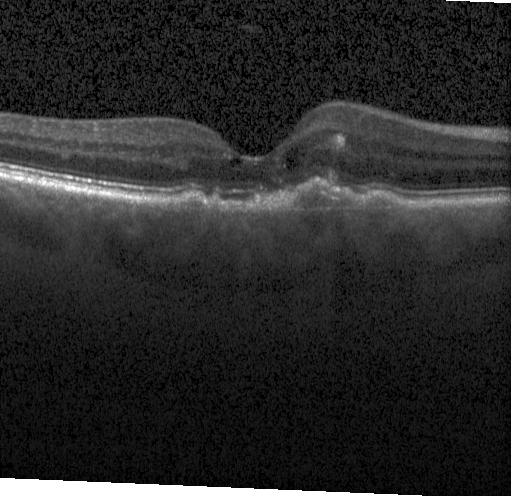 Centered on the fovea. SD-OCT. OCT line scan. Acquired on a Heidelberg Spectralis
The scan shows choroidal neovascularization (CNV).